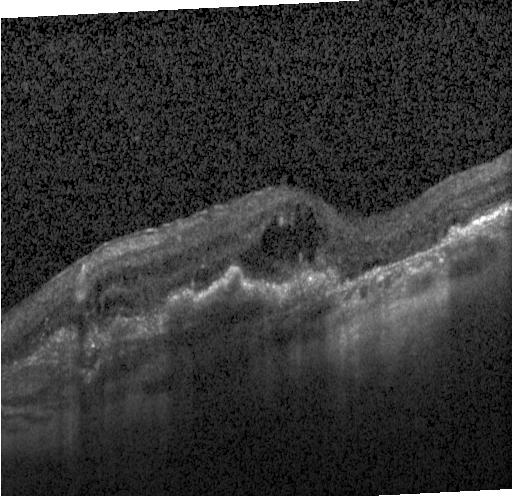
Impression: a choroidal neovascular membrane.